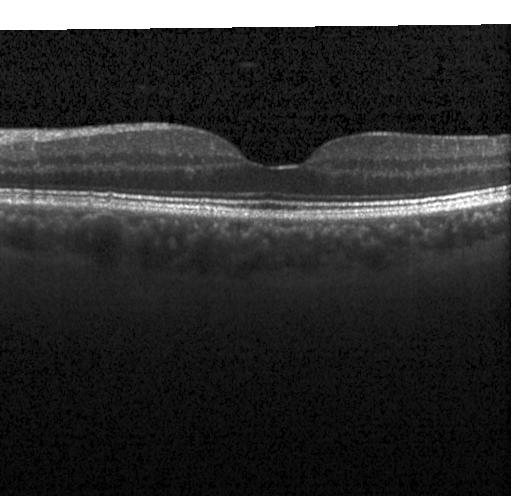

OCT line scan · spectral-domain optical coherence tomography · fovea-centered
Macular OCT: no CNV, no DME, and no drusen.